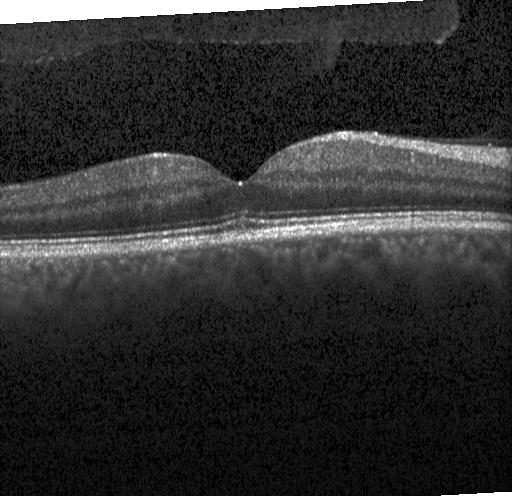
Optical coherence tomography B-scan, through the macula.
This B-scan demonstrates neither choroidal neovascularization, diabetic macular edema, nor drusen.